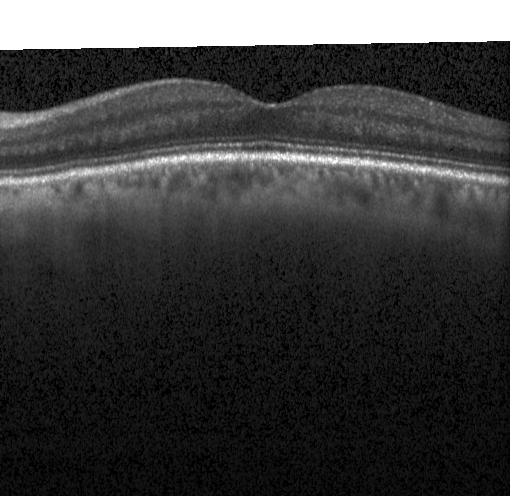

Heidelberg Spectralis OCT system · spectral-domain optical coherence tomography · retinal OCT B-scan · macular scan
This B-scan demonstrates no choroidal neovascularization, diabetic macular edema, or drusen.